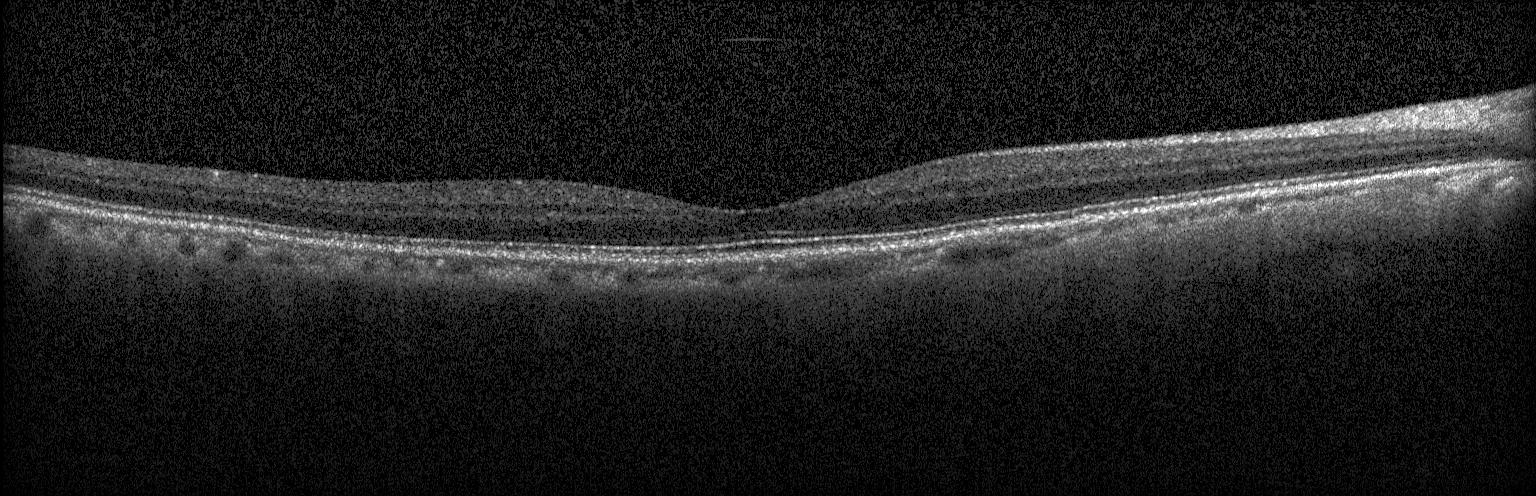
Retinal OCT cross-section, spectral-domain OCT.
OCT finding: neither CNV, DME, nor drusen.